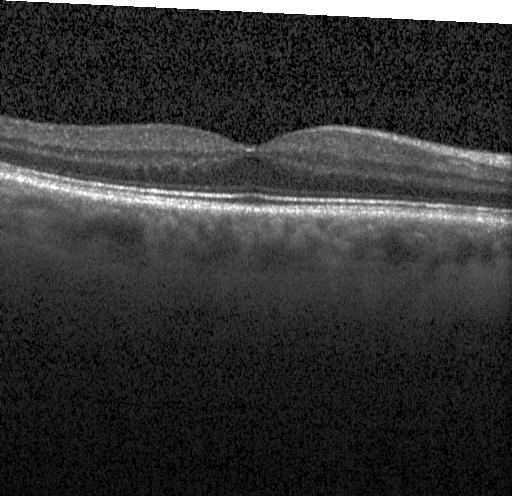

OCT B-scan. Macular scan. Spectral-domain OCT. This B-scan demonstrates no evidence of choroidal neovascularization, diabetic macular edema, or drusen.